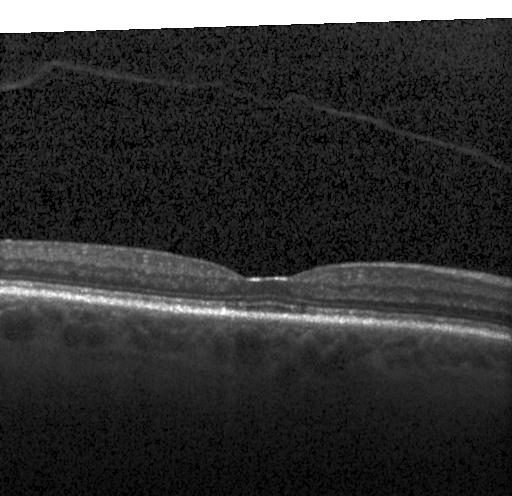
Diagnosis: neither choroidal neovascularization, diabetic macular edema, nor drusen.